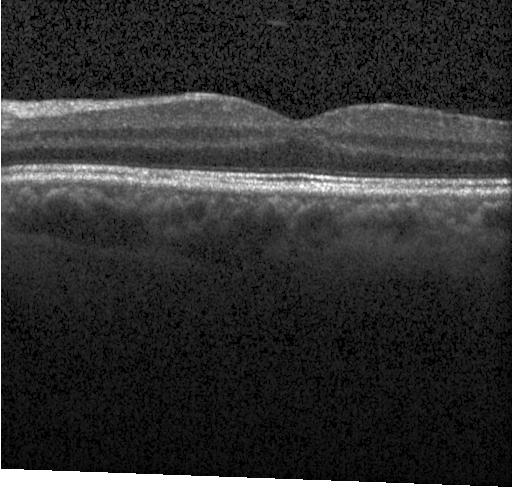
Optical coherence tomography B-scan. Instrument: Heidelberg Spectralis. Through the macula. Spectral-domain OCT — OCT finding: neither choroidal neovascularization, diabetic macular edema, nor drusen.